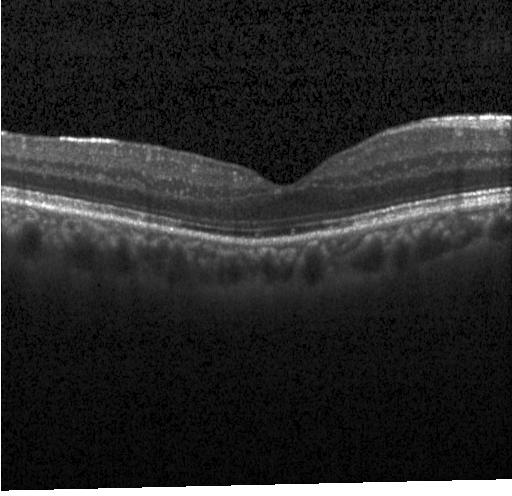 SD-OCT, through the macula, instrument: Heidelberg Spectralis, retinal OCT B-scan.
The scan shows no evidence of choroidal neovascularization, diabetic macular edema, or drusen.